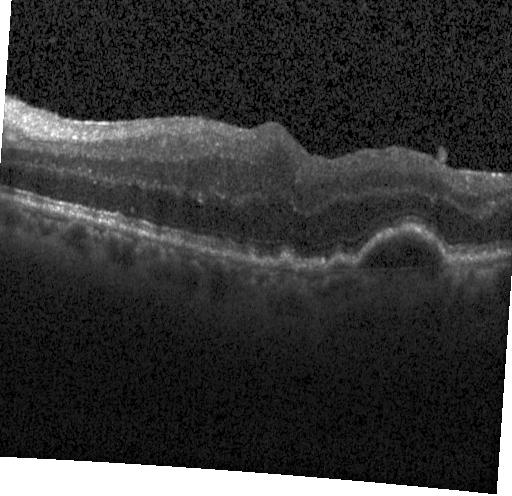 Centered on the fovea. Retinal OCT cross-section. SD-OCT
Macular OCT: choroidal neovascularization (CNV).